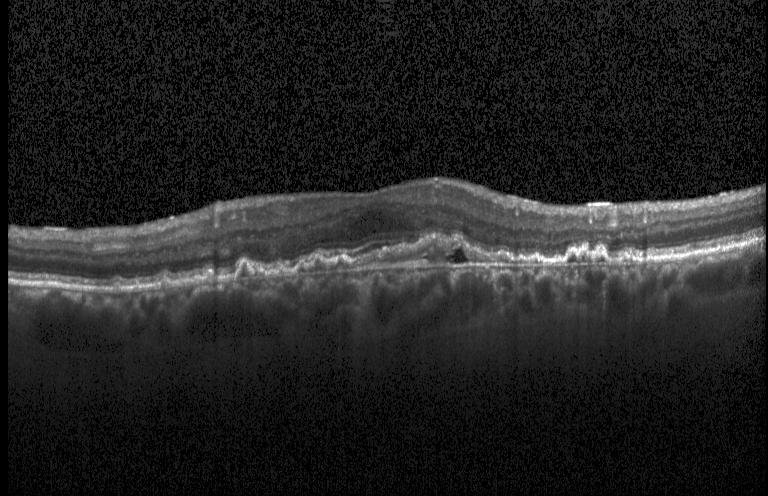 Retinal OCT B-scan; Heidelberg Spectralis OCT system
Dx: choroidal neovascularization (CNV).